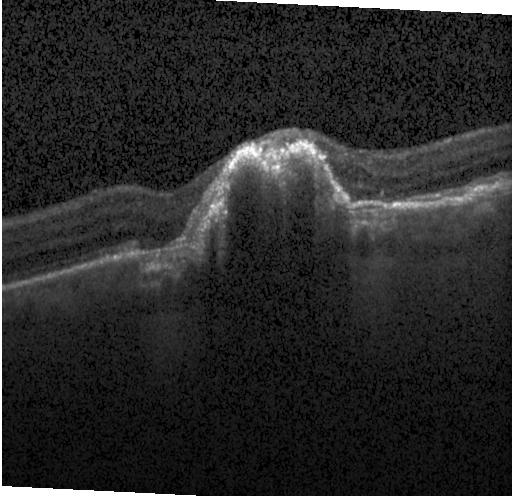
Optical coherence tomography scan, macular scan
CNV.